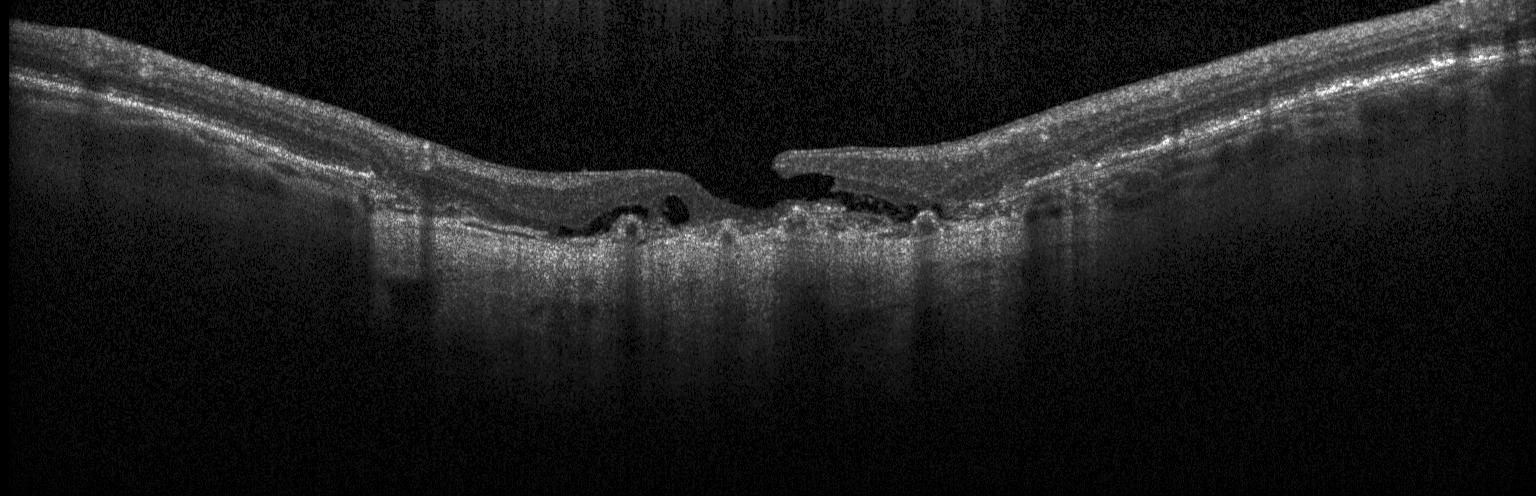

OCT finding: a choroidal neovascular membrane.